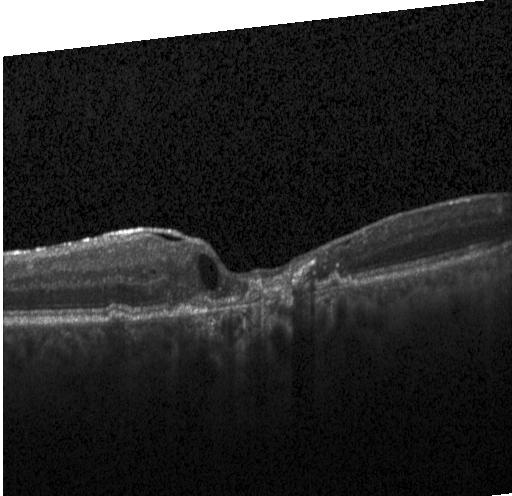
OCT B-scan showing choroidal neovascularization.